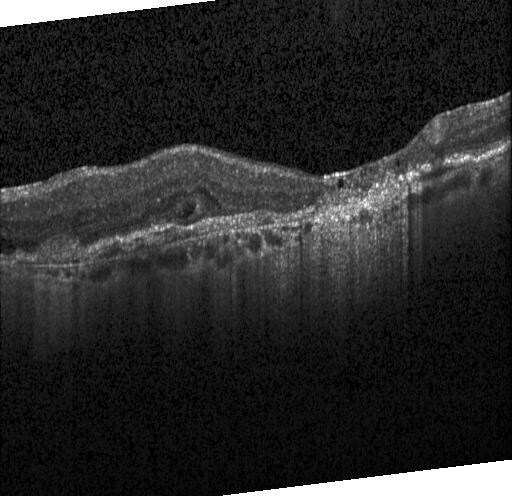

Heidelberg Spectralis OCT system · spectral-domain optical coherence tomography · OCT B-scan.
Diagnosis: choroidal neovascularization (CNV).